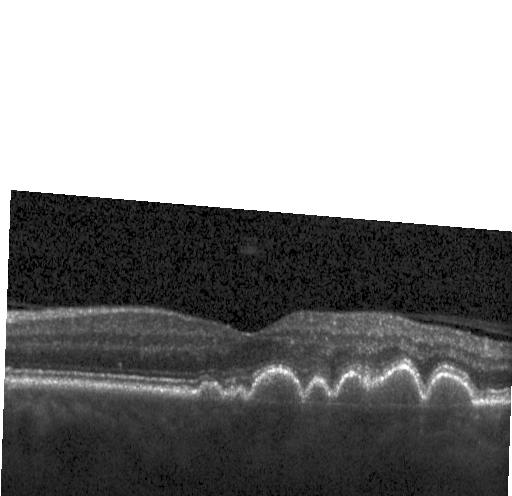
Heidelberg Spectralis; SD-OCT; OCT B-scan.
Dx: drusen.